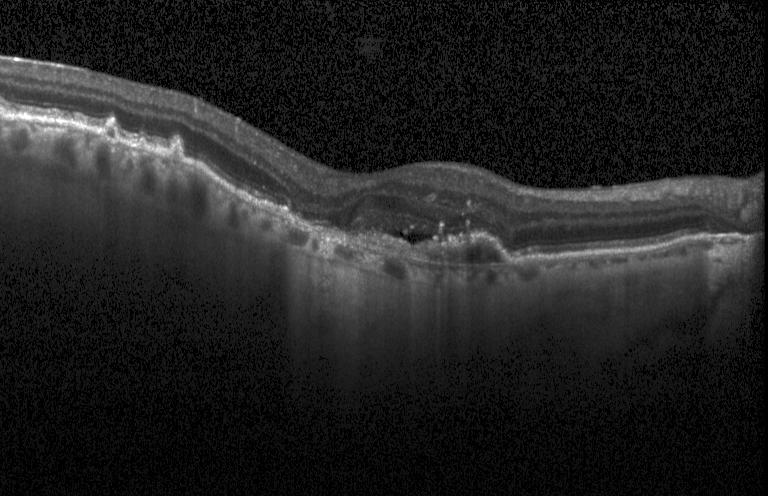
OCT B-scan. Spectral-domain optical coherence tomography. Instrument: Heidelberg Spectralis — Diagnosis: choroidal neovascularization.